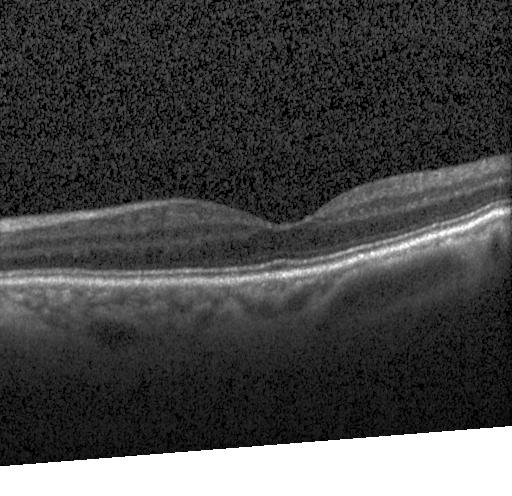
OCT B-scan
No choroidal neovascularization, diabetic macular edema, or drusen.